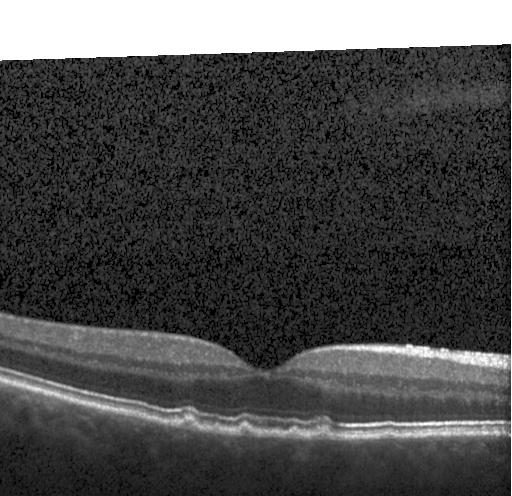 Diagnosis: multiple drusen.